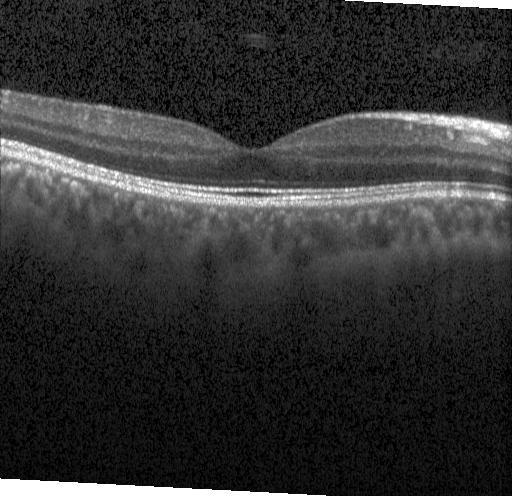

Optical coherence tomography scan
Macular OCT: no evidence of choroidal neovascularization, diabetic macular edema, or drusen.